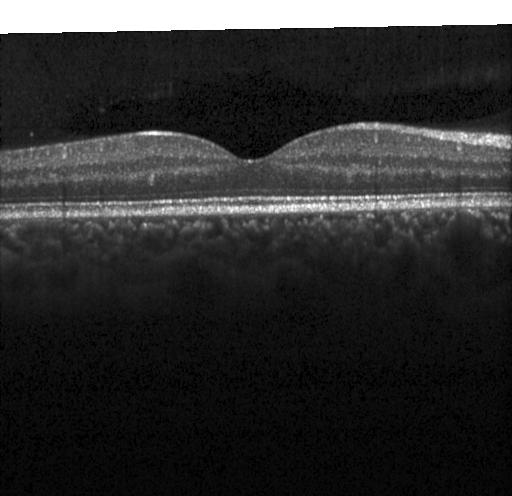

OCT line scan; acquired on a Heidelberg Spectralis. Finding: no choroidal neovascularization, no diabetic macular edema, and no drusen.